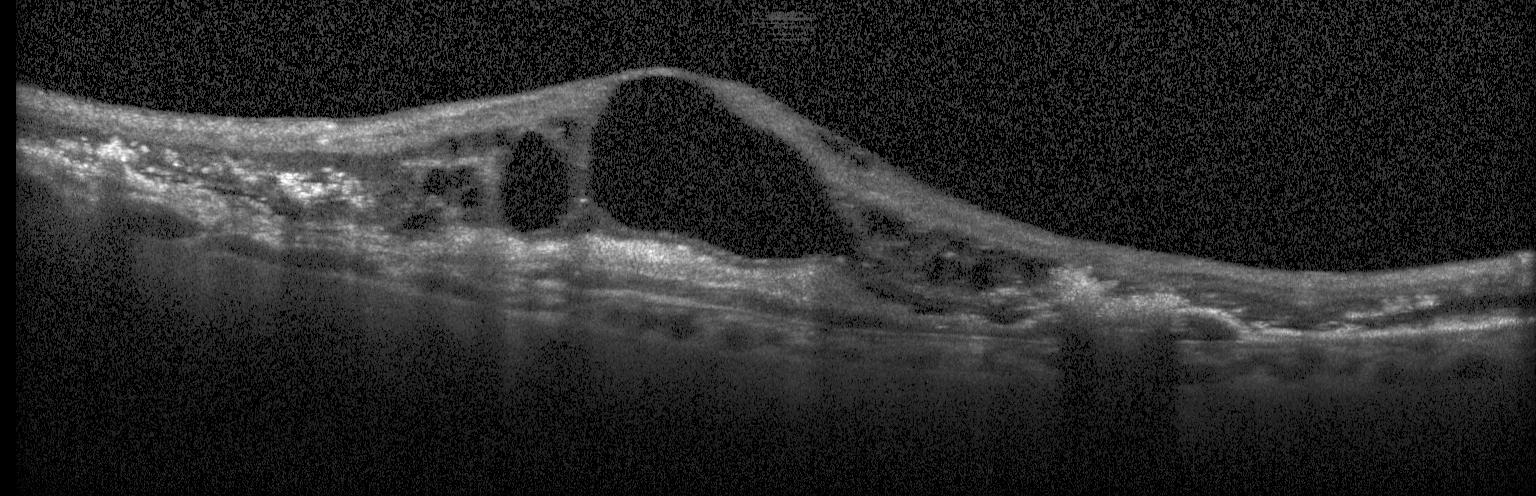
OCT line scan; SD-OCT; horizontal scan through the fovea
Diagnosis: CNV.